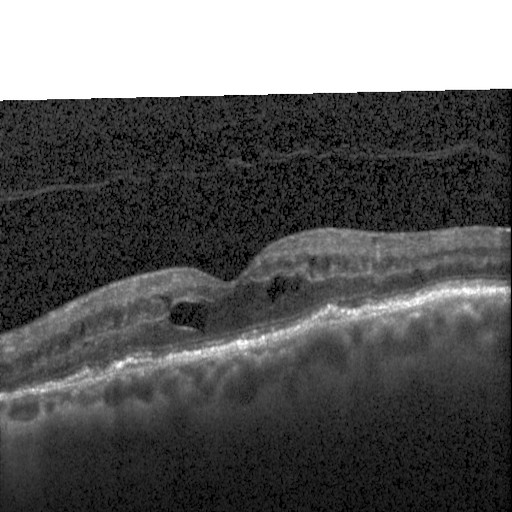 Retinal OCT cross-section.
Impression: diabetic macular edema (DME).